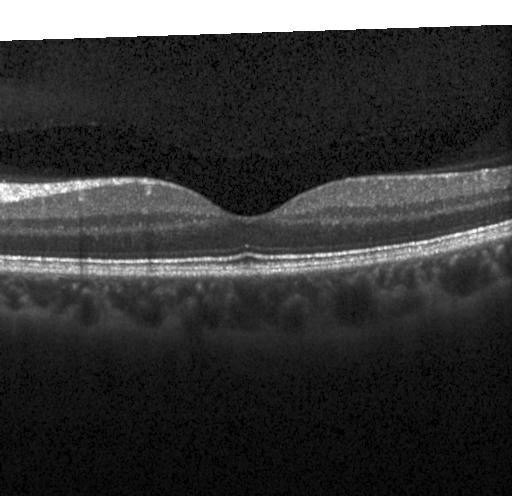 Spectral-domain OCT · OCT B-scan.
Diagnosis: no evidence of choroidal neovascularization, diabetic macular edema, or drusen.